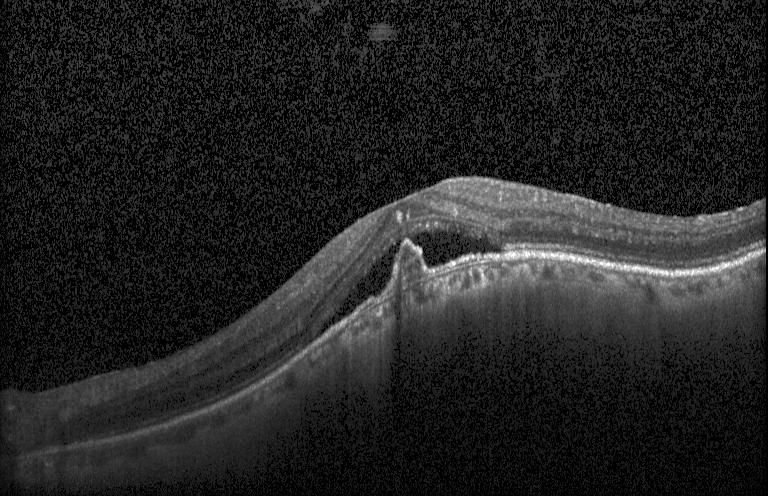 Acquired on a Heidelberg Spectralis. Macular scan. Retinal OCT cross-section. Spectral-domain optical coherence tomography
Impression: a choroidal neovascular membrane.